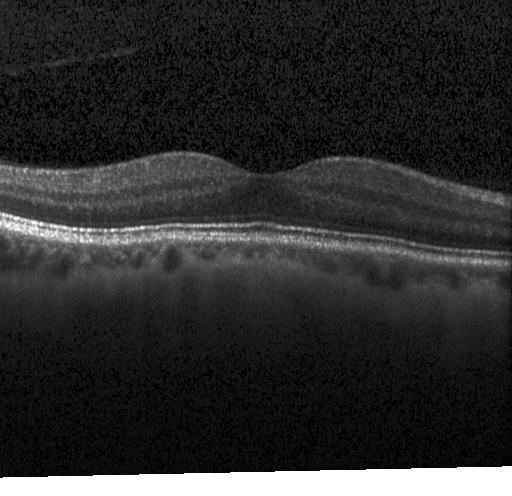
Finding: no CNV, no DME, and no drusen.